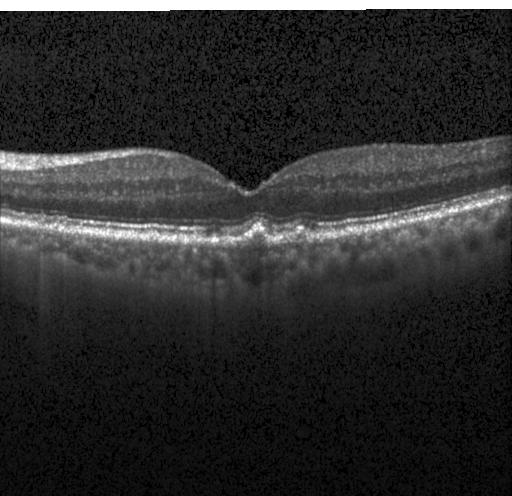

SD-OCT. OCT B-scan. Centered on the fovea
Finding: sub-RPE drusenoid deposits.